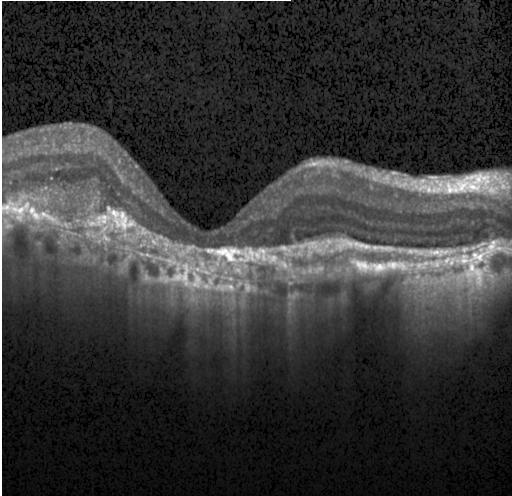
Diagnosis: a choroidal neovascular membrane.